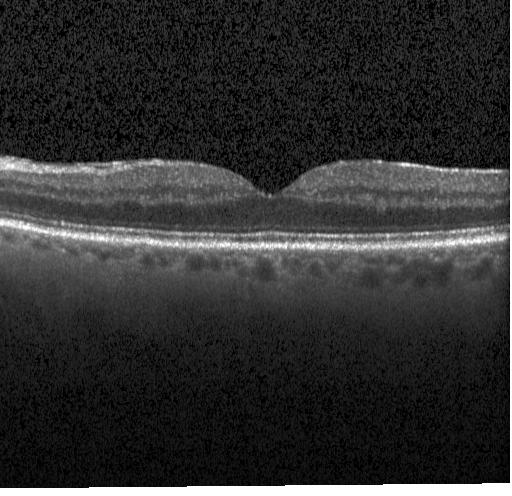
OCT line scan. Diagnosis: neither CNV, DME, nor drusen.